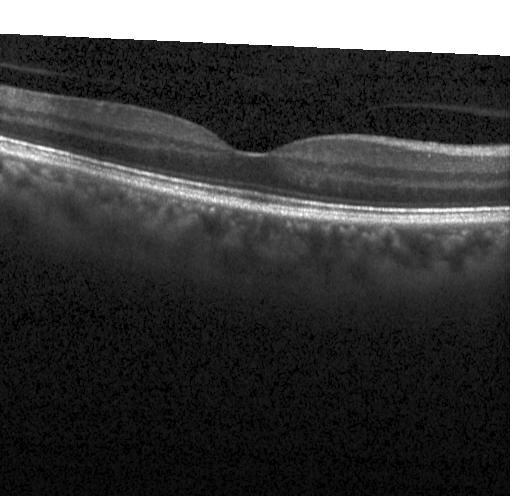 Horizontal scan through the fovea; instrument: Heidelberg Spectralis; SD-OCT; optical coherence tomography B-scan.
Finding: no evidence of choroidal neovascularization, diabetic macular edema, or drusen.